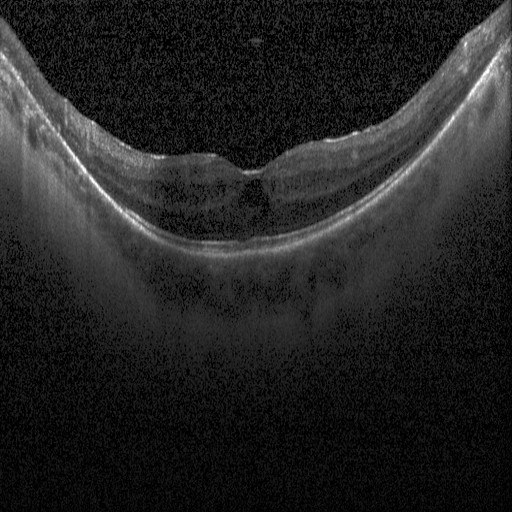
Retinal OCT cross-section. Spectral-domain optical coherence tomography.
Dx: diabetic macular edema.